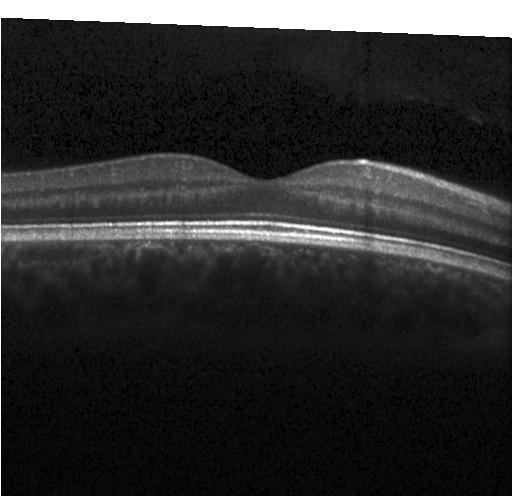 Retinal OCT cross-section. Impression: neither choroidal neovascularization, diabetic macular edema, nor drusen.